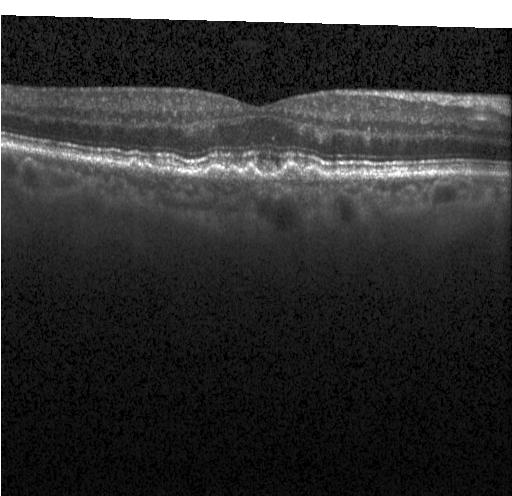

Through the macula, SD-OCT, retinal OCT cross-section, acquired on a Heidelberg Spectralis
Impression: drusen.